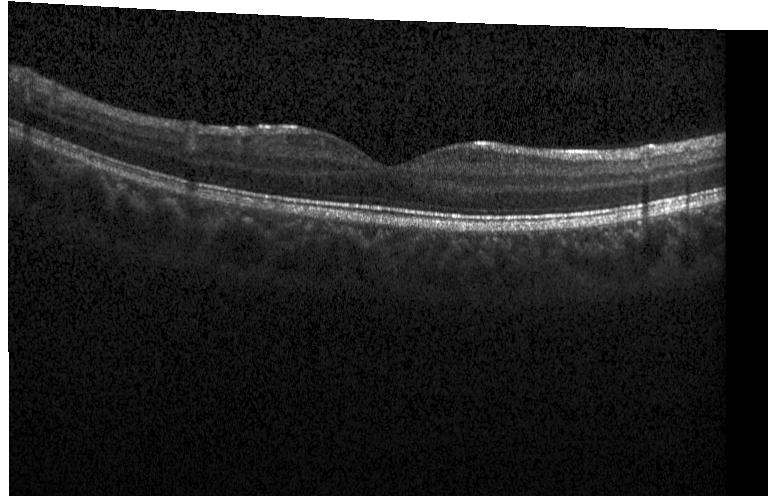 The scan shows neither choroidal neovascularization, diabetic macular edema, nor drusen.